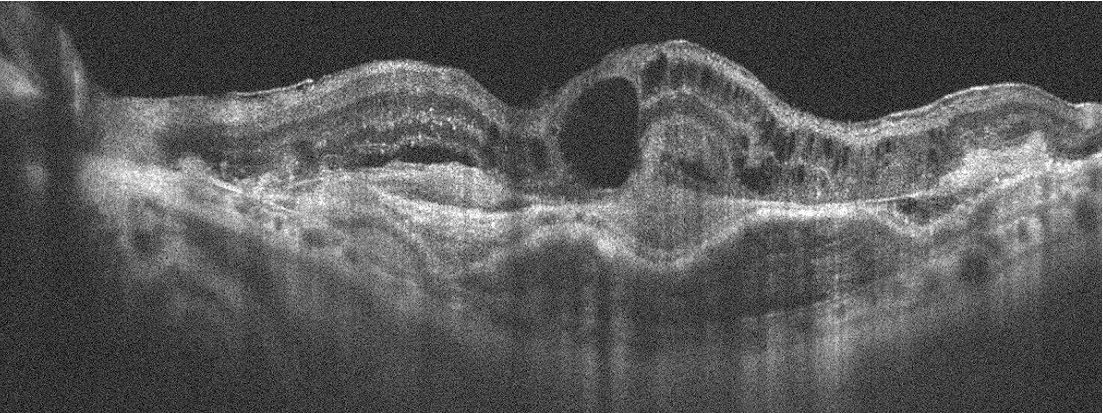
Finding: age-related macular degeneration.